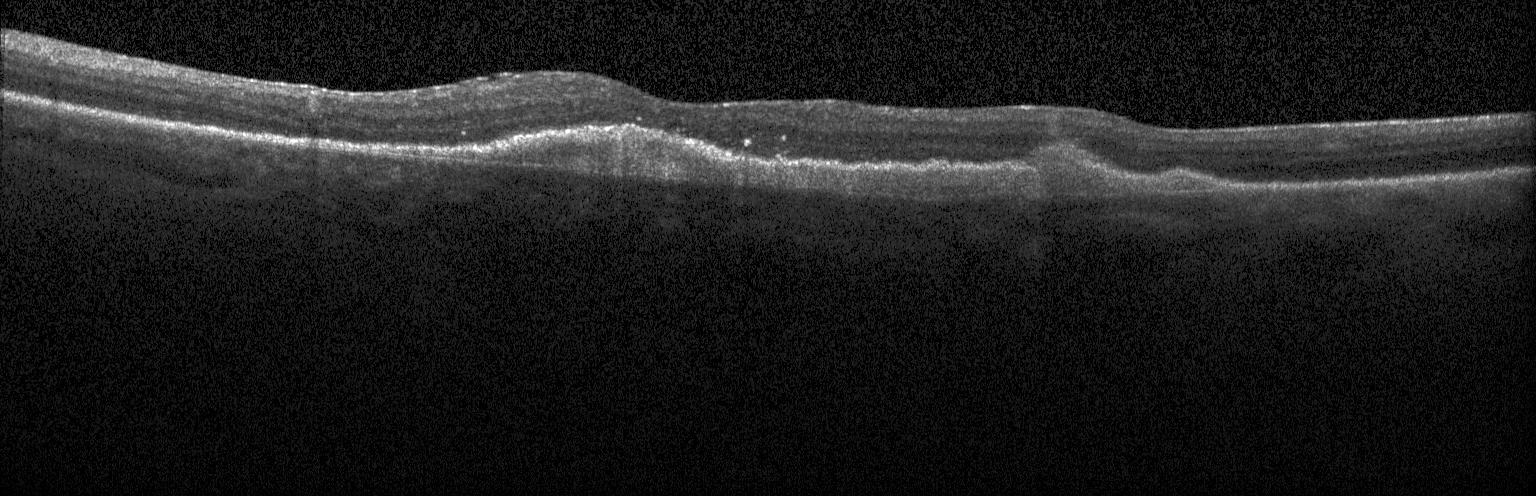
Optical coherence tomography B-scan.
Finding: a choroidal neovascular membrane.